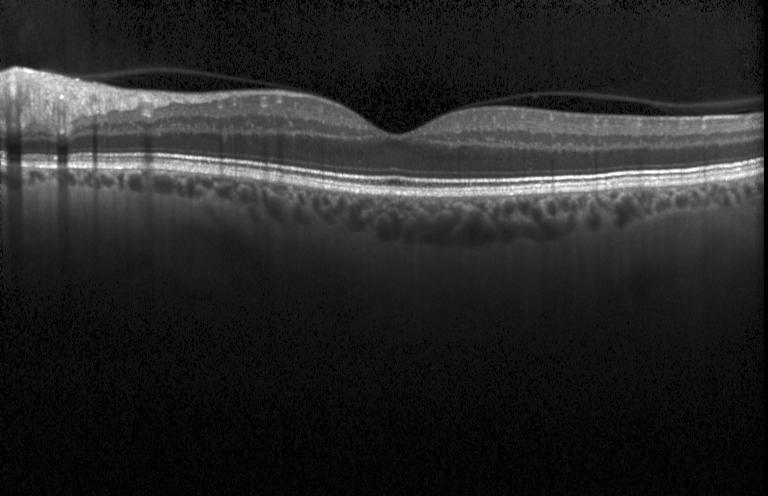
Macular OCT: no evidence of choroidal neovascularization, diabetic macular edema, or drusen.